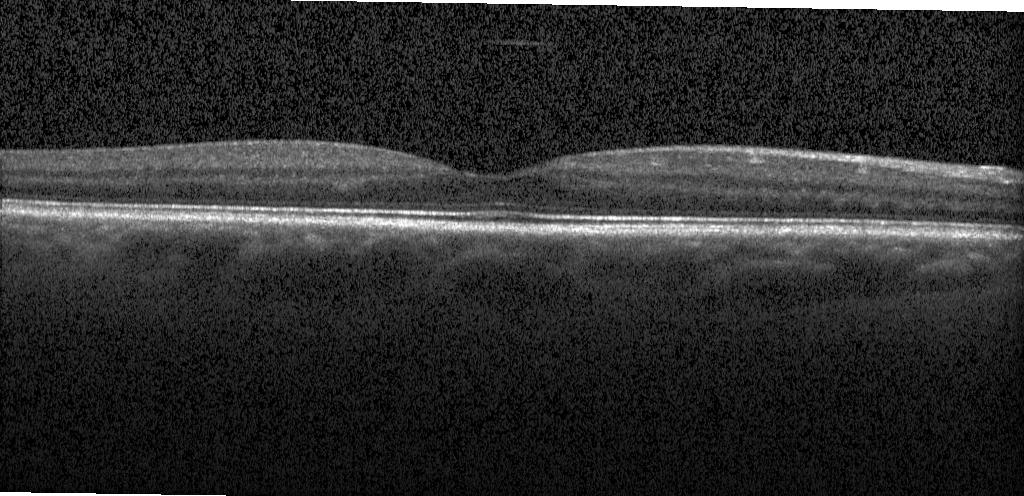 Macular OCT demonstrating no CNV, DME, or drusen.